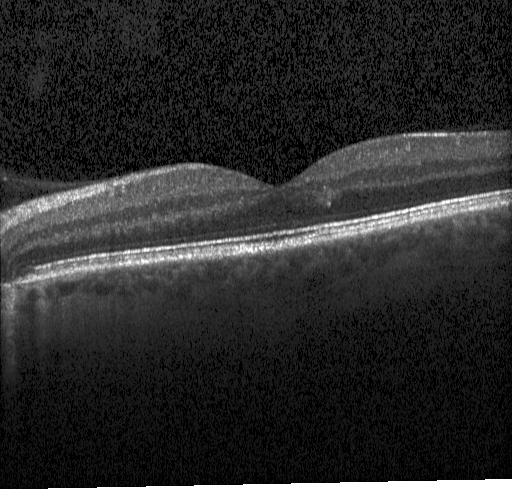

Through the macula · optical coherence tomography B-scan · Heidelberg Spectralis OCT system. The scan shows neither CNV, DME, nor drusen.